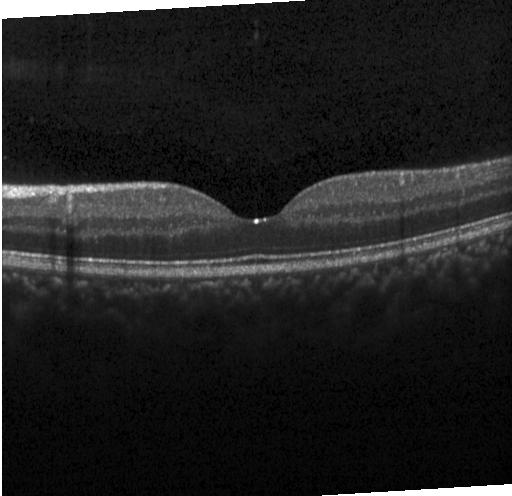
The scan shows no CNV, DME, or drusen.